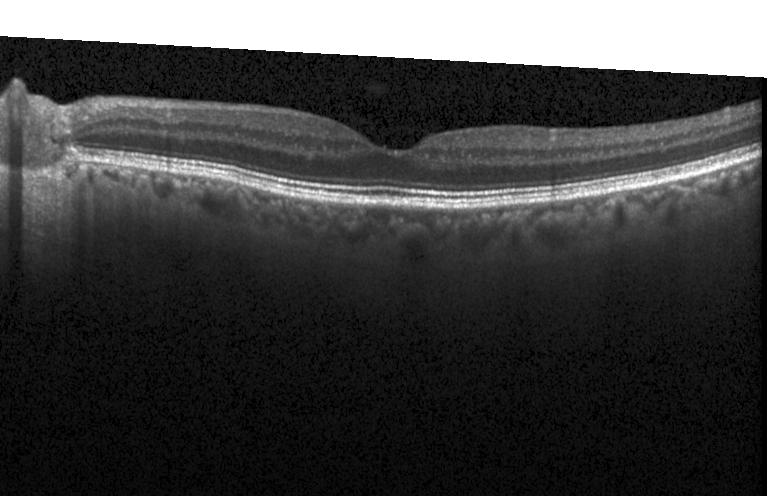

The scan shows no CNV, no DME, and no drusen.